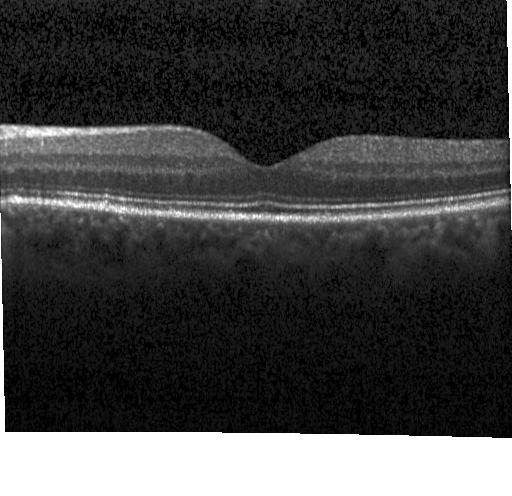

SD-OCT; instrument: Heidelberg Spectralis; retinal OCT cross-section.
Finding: neither choroidal neovascularization, diabetic macular edema, nor drusen.